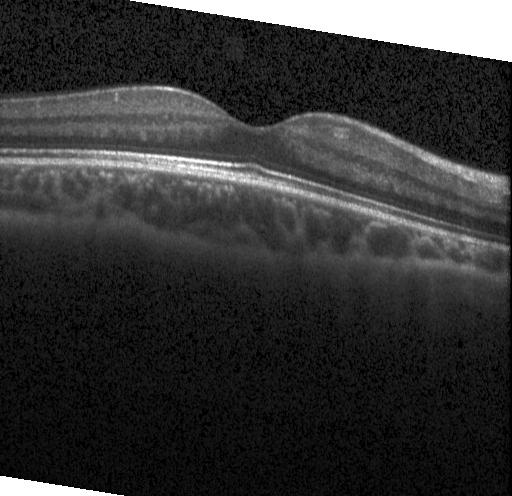
Optical coherence tomography B-scan. Diagnosis: no choroidal neovascularization, diabetic macular edema, or drusen.